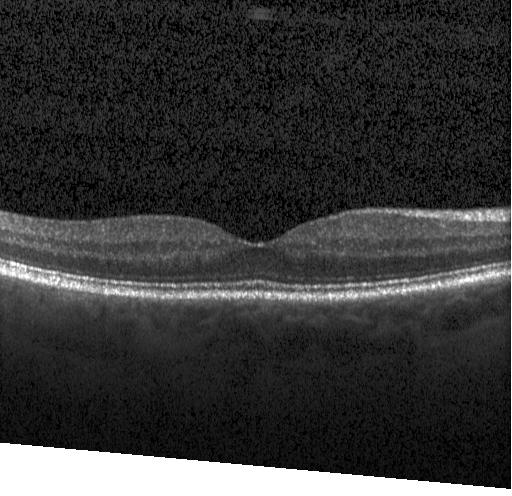 Optical coherence tomography scan. OCT finding: no choroidal neovascularization, no diabetic macular edema, and no drusen.